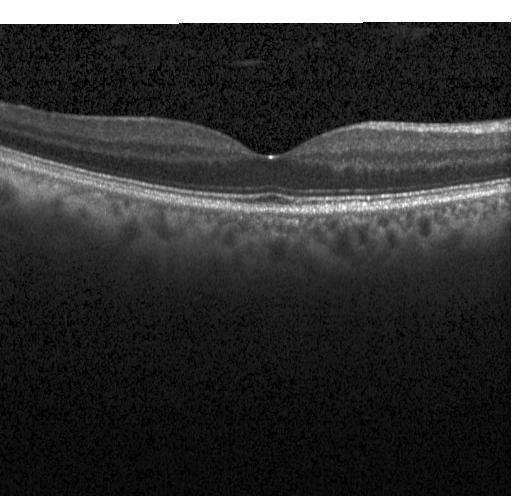
Acquired on a Heidelberg Spectralis; optical coherence tomography B-scan; macular scan. Impression: no evidence of choroidal neovascularization, diabetic macular edema, or drusen.